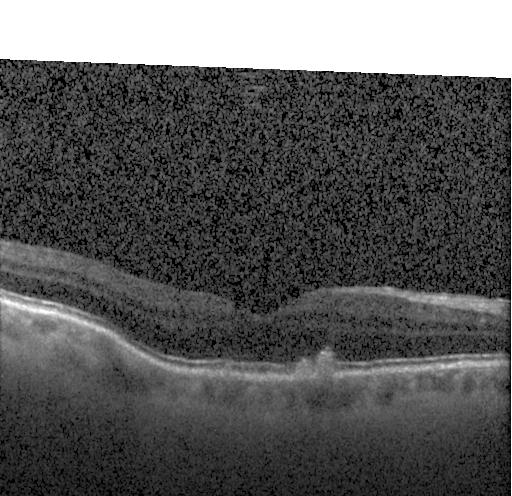
Retinal OCT B-scan, horizontal scan through the fovea. This B-scan demonstrates sub-RPE drusenoid deposits.